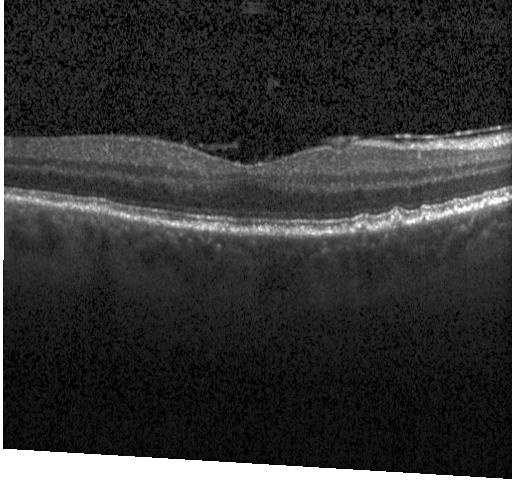
Retinal OCT B-scan
Impression: sub-RPE drusenoid deposits.